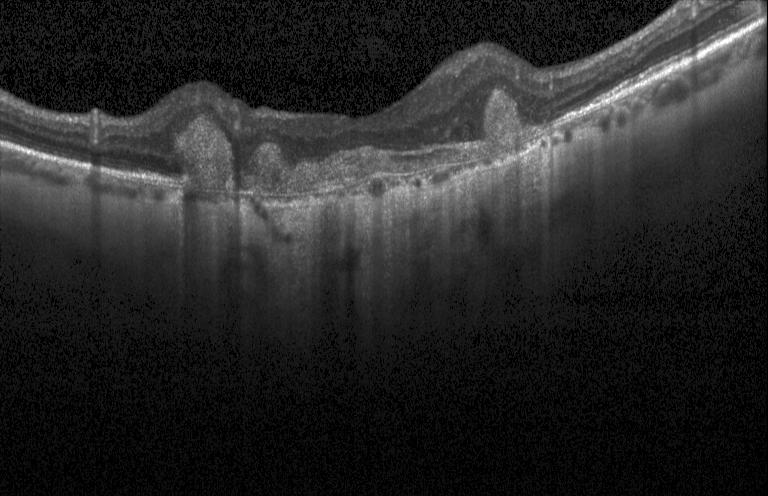
Assessment: choroidal neovascularization.